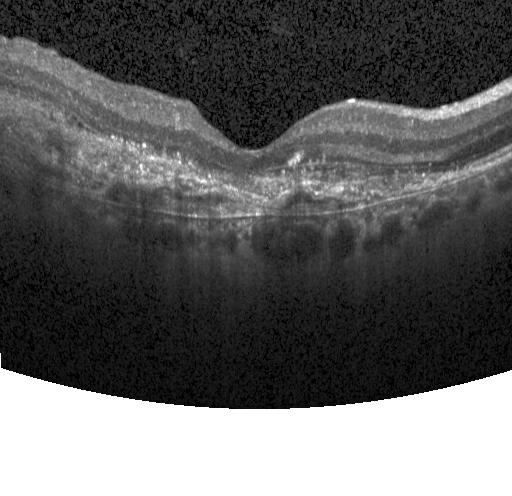
Impression: a choroidal neovascular membrane.